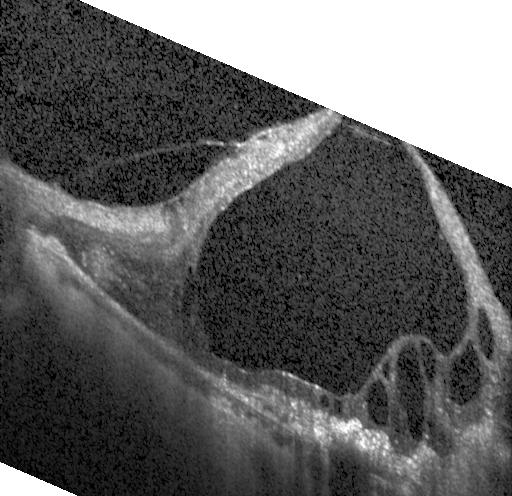
Centered on the fovea; acquired on a Heidelberg Spectralis; optical coherence tomography B-scan; spectral-domain optical coherence tomography
This B-scan demonstrates a choroidal neovascular membrane.